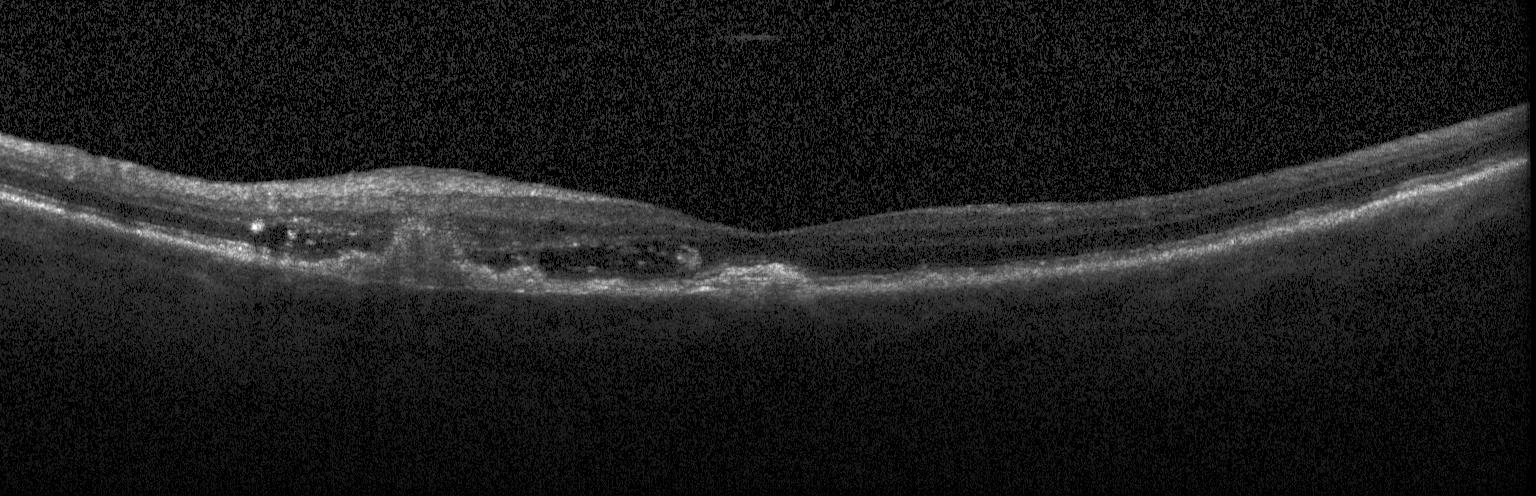

Impression: a choroidal neovascular membrane.